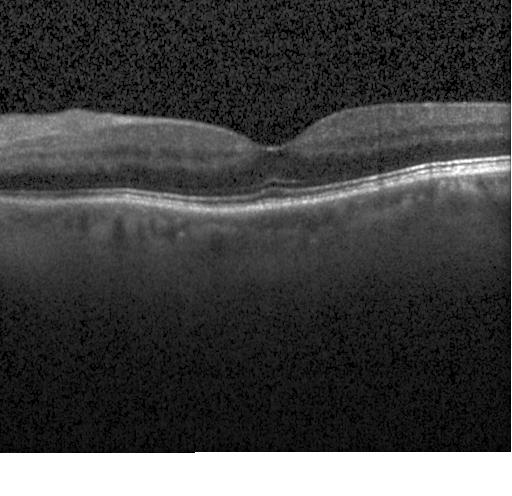

Fovea-centered; optical coherence tomography B-scan — Finding: no choroidal neovascularization, no diabetic macular edema, and no drusen.